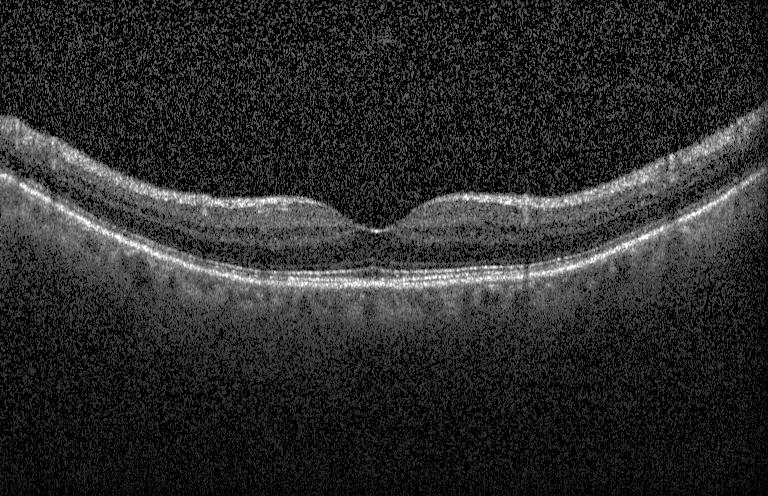

Finding: no choroidal neovascularization, no diabetic macular edema, and no drusen.